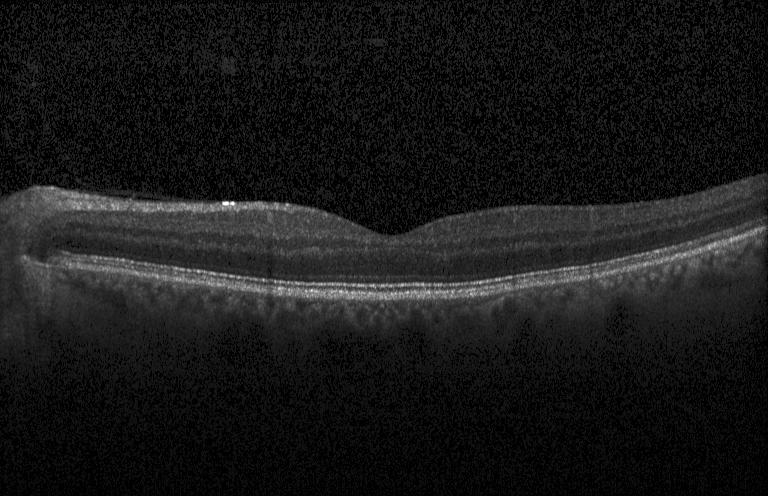

Finding: no CNV, no DME, and no drusen.